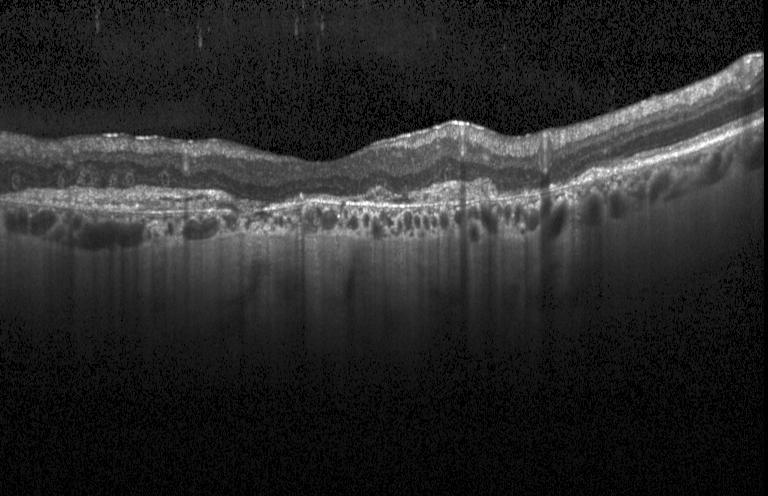
SD-OCT, instrument: Heidelberg Spectralis, centered on the fovea, OCT B-scan.
Assessment: a choroidal neovascular membrane.